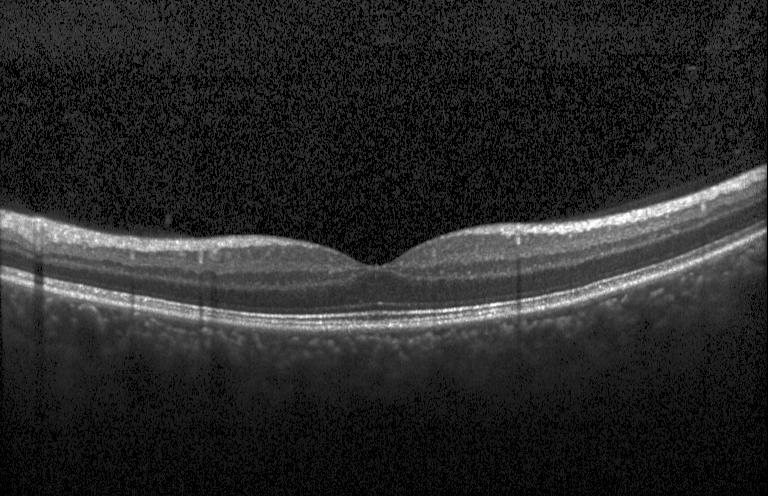
Impression: no choroidal neovascularization, no diabetic macular edema, and no drusen.